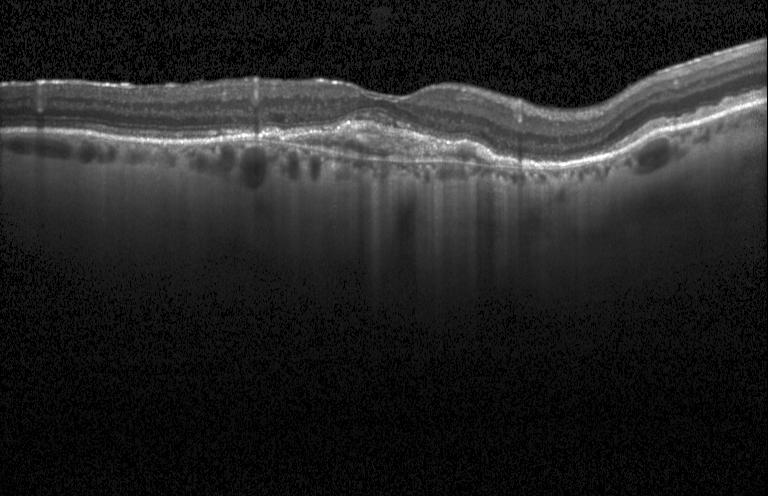 Retinal OCT cross-section — Macular OCT: a choroidal neovascular membrane.